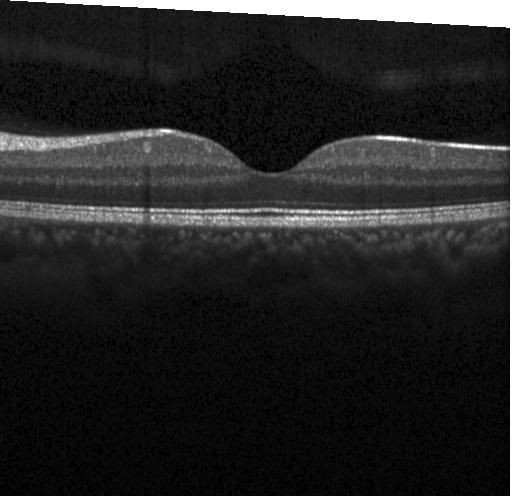
Heidelberg Spectralis; centered on the fovea; spectral-domain OCT; retinal OCT B-scan
Finding: neither CNV, DME, nor drusen.